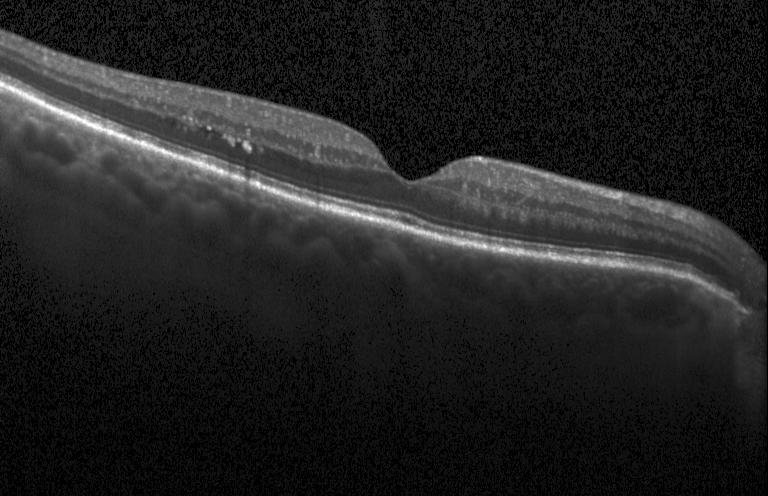 The scan shows no choroidal neovascularization, diabetic macular edema, or drusen.